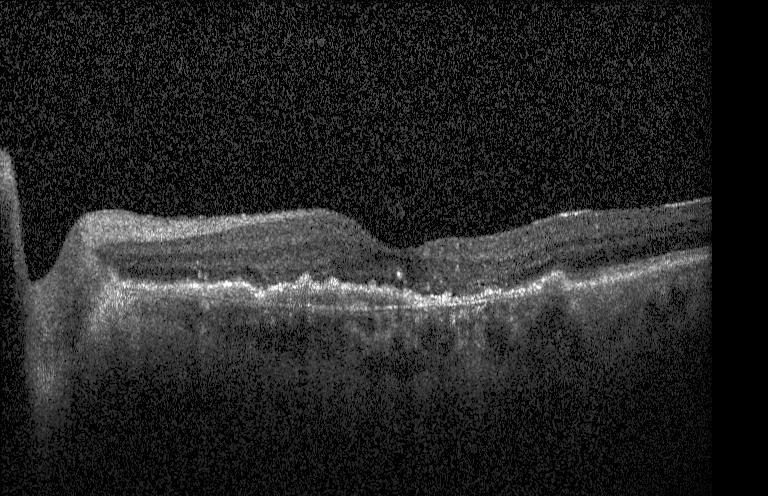 Heidelberg Spectralis OCT system. Retinal OCT cross-section.
Diagnosis: choroidal neovascularization (CNV).